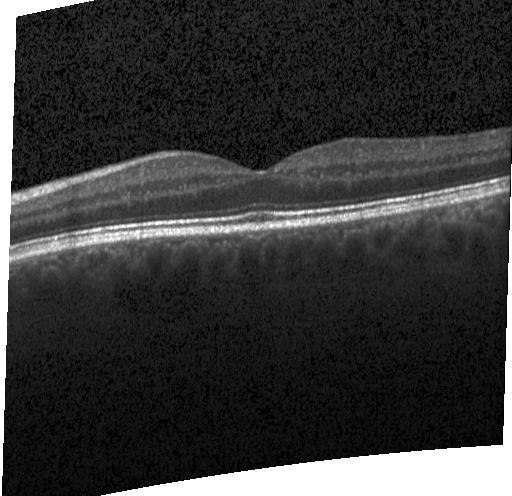 Centered on the fovea. Retinal OCT B-scan. Heidelberg Spectralis. Spectral-domain optical coherence tomography. Impression: neither choroidal neovascularization, diabetic macular edema, nor drusen.